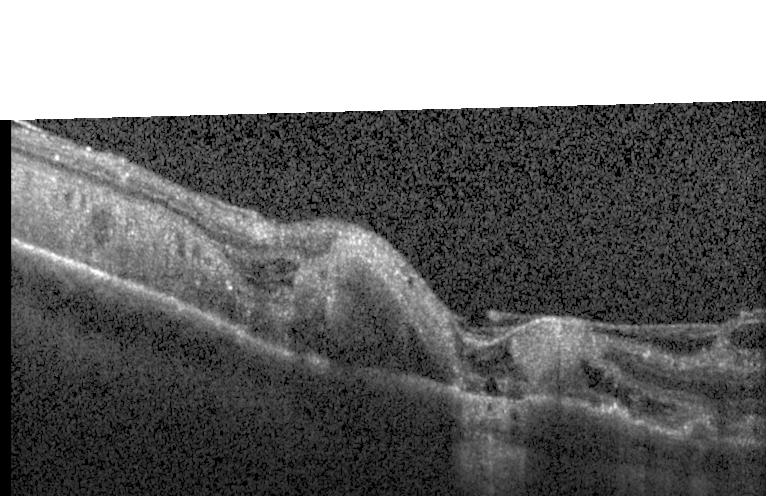
Optical coherence tomography B-scan
Choroidal neovascularization.